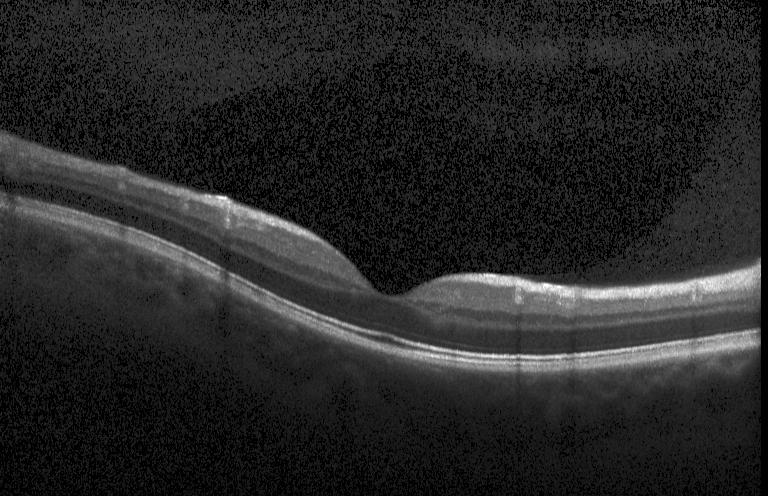

Macular OCT demonstrating no choroidal neovascularization, no diabetic macular edema, and no drusen.